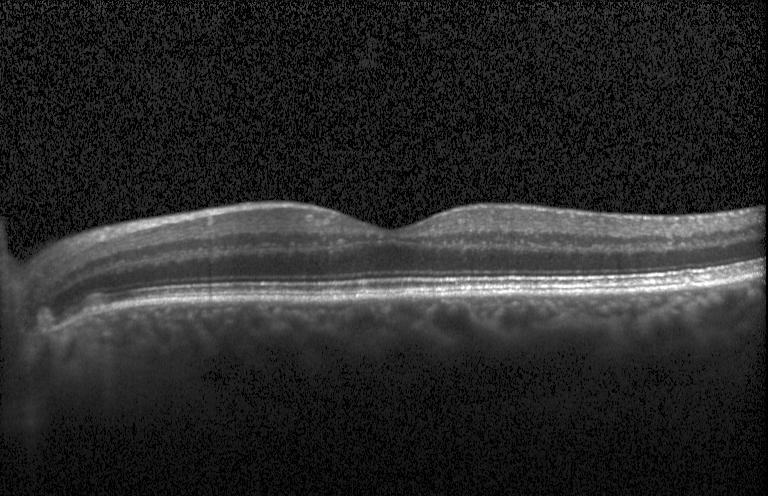
Spectral-domain optical coherence tomography; retinal OCT B-scan; instrument: Heidelberg Spectralis; macular scan.
Impression: no choroidal neovascularization, no diabetic macular edema, and no drusen.